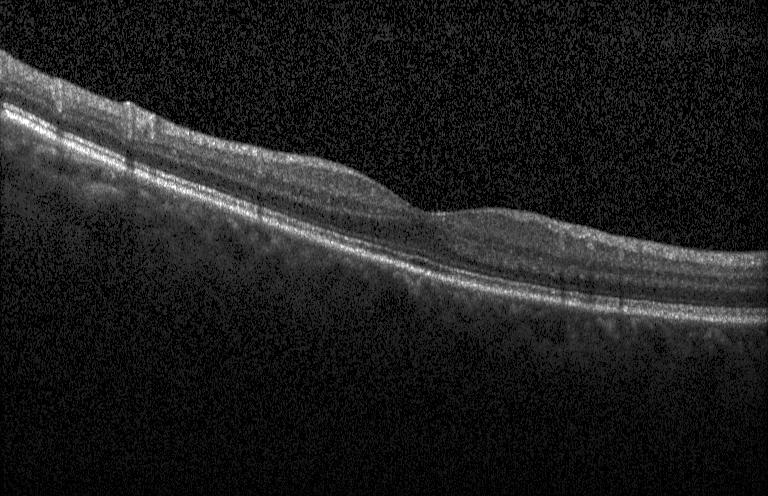

Optical coherence tomography B-scan.
Dx: neither choroidal neovascularization, diabetic macular edema, nor drusen.